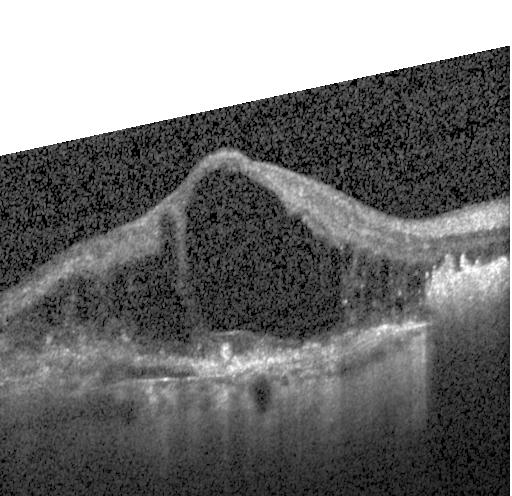 Retinal OCT cross-section · instrument: Heidelberg Spectralis. Assessment: choroidal neovascularization.